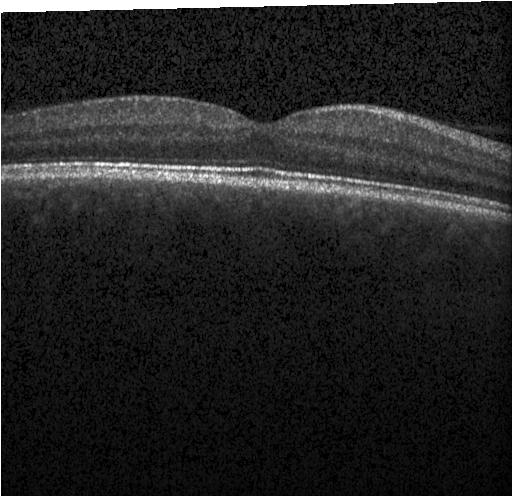

Centered on the fovea · optical coherence tomography B-scan
Impression: no CNV, no DME, and no drusen.